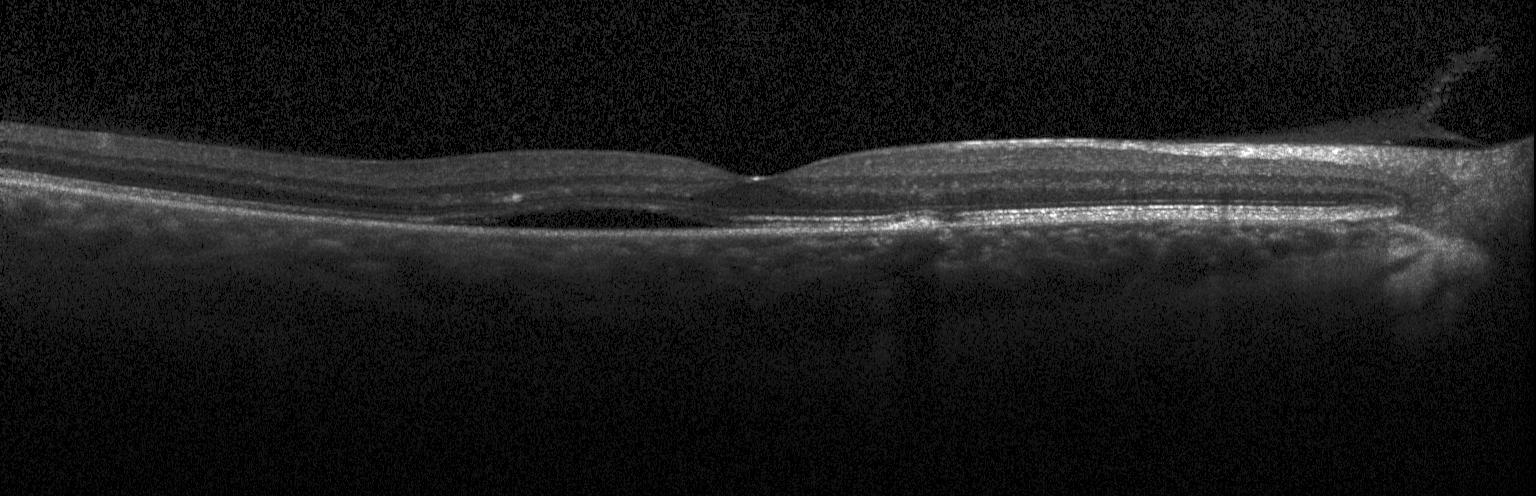
Macular OCT: a choroidal neovascular membrane.